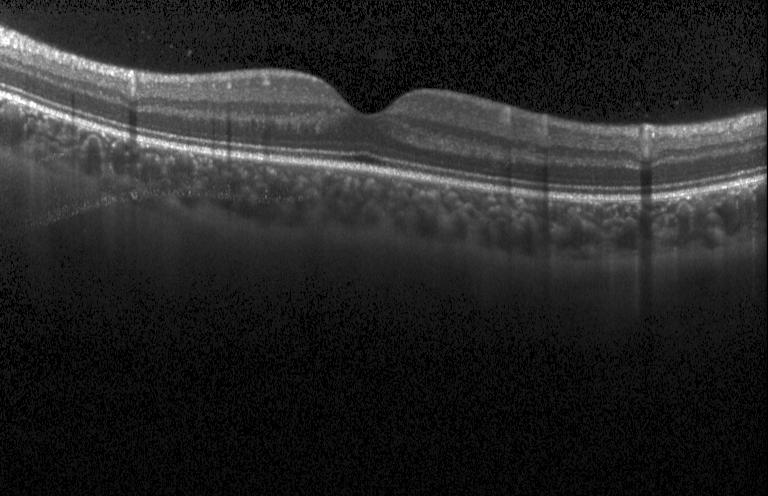

Acquired on a Heidelberg Spectralis · OCT B-scan — Finding: no choroidal neovascularization, no diabetic macular edema, and no drusen.